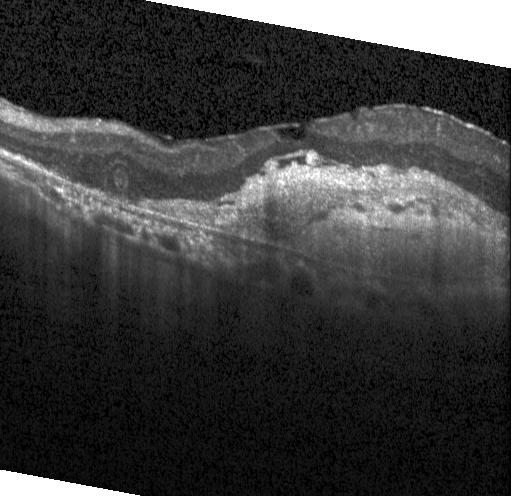 Retinal OCT B-scan, Heidelberg Spectralis, fovea-centered — A choroidal neovascular membrane.